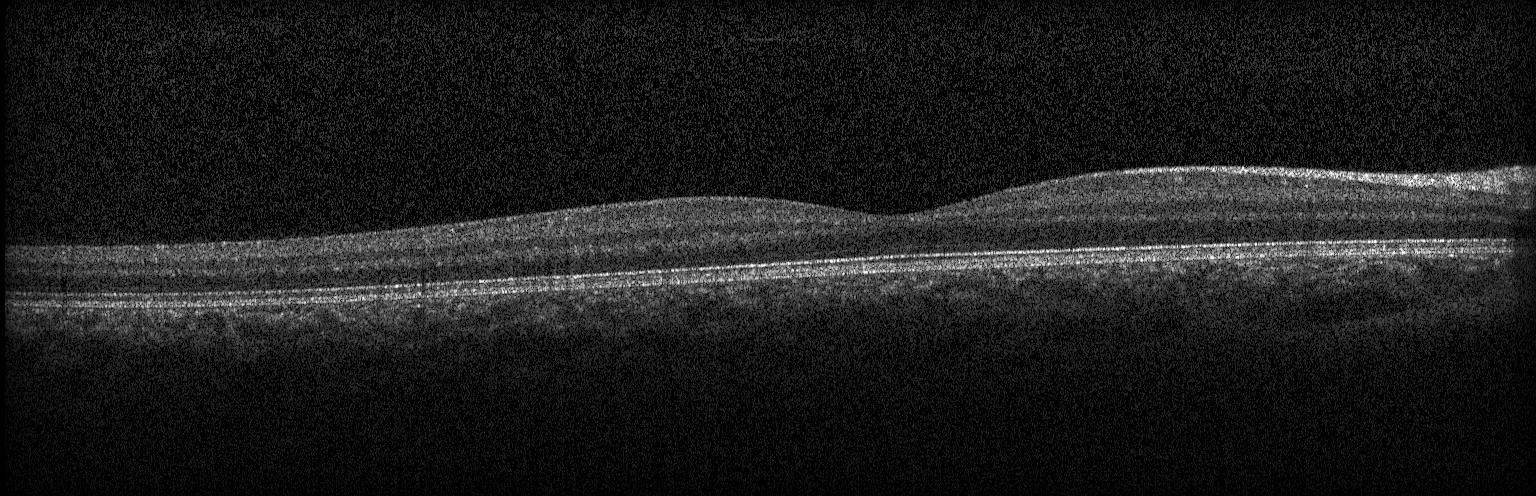

Heidelberg Spectralis. Optical coherence tomography scan. Horizontal scan through the fovea.
Dx: no evidence of CNV, DME, or drusen.